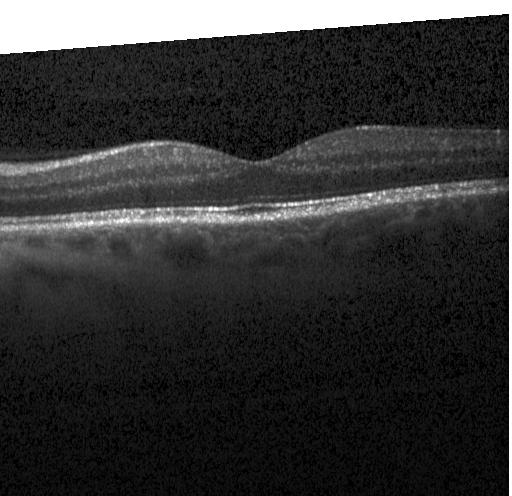 Optical coherence tomography B-scan
Finding: no evidence of choroidal neovascularization, diabetic macular edema, or drusen.